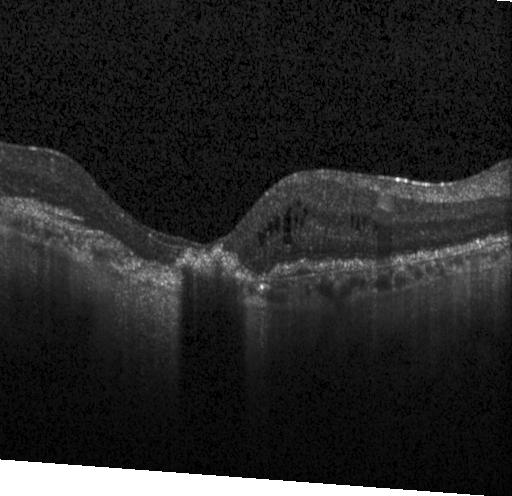 SD-OCT · retinal OCT B-scan · fovea-centered · acquired on a Heidelberg Spectralis — This B-scan demonstrates a choroidal neovascular membrane.